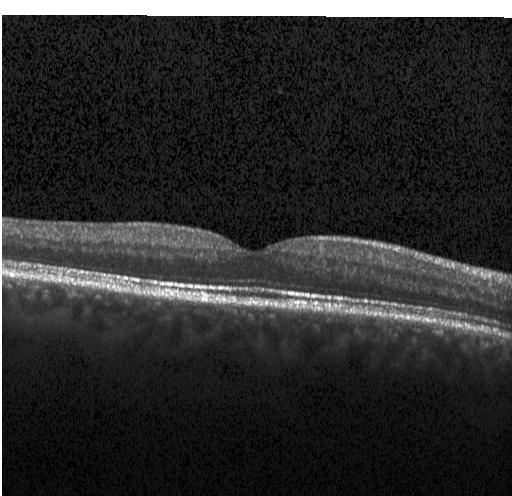
SD-OCT · OCT line scan. Dx: no evidence of choroidal neovascularization, diabetic macular edema, or drusen.